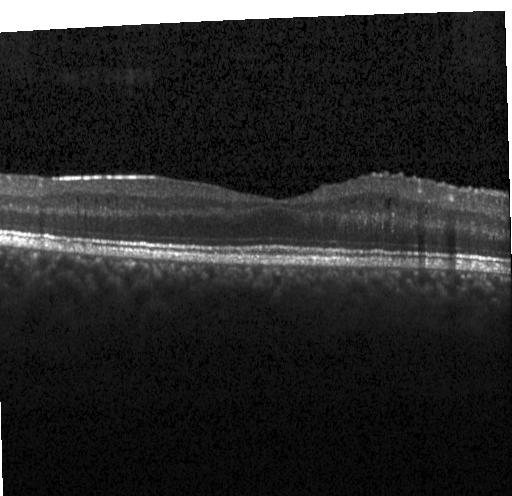

Heidelberg Spectralis OCT system · retinal OCT B-scan — Dx: diabetic macular edema.